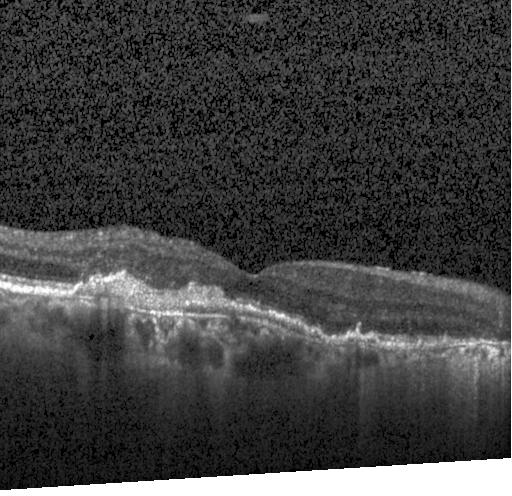
Optical coherence tomography scan, SD-OCT, Heidelberg Spectralis.
Macular OCT: CNV.